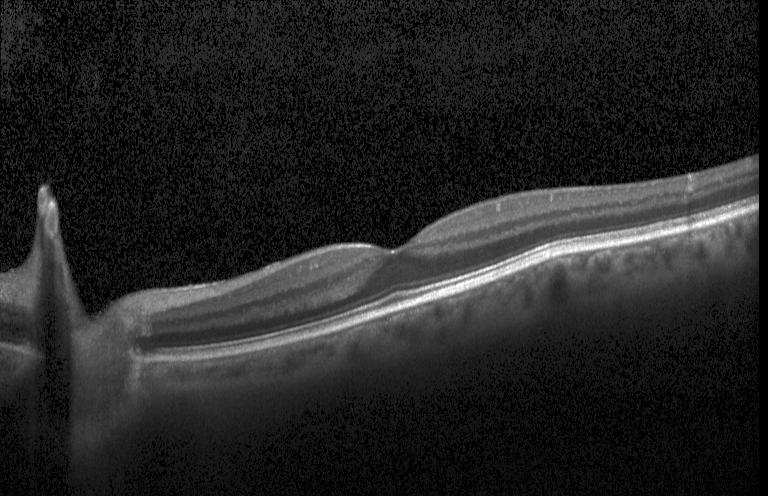

Macular OCT demonstrating no CNV, DME, or drusen.